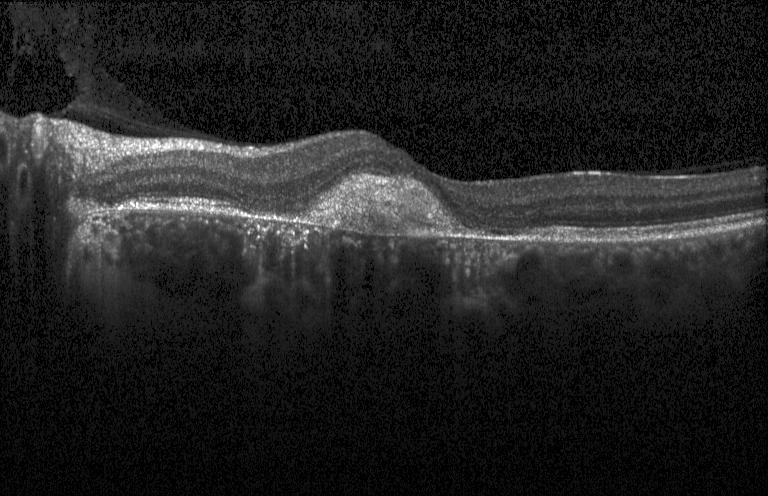

A choroidal neovascular membrane.